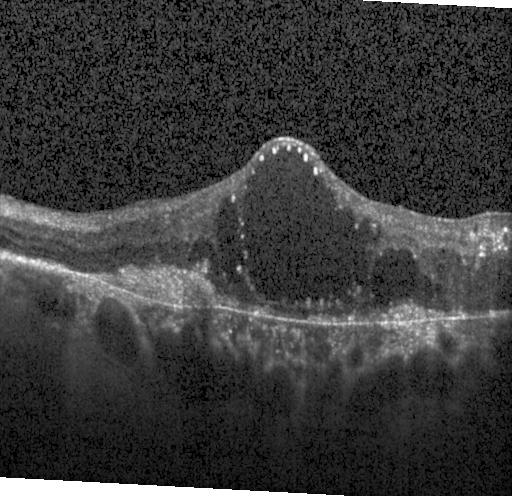

Acquired on a Heidelberg Spectralis; macular scan; OCT B-scan
Dx: CNV.